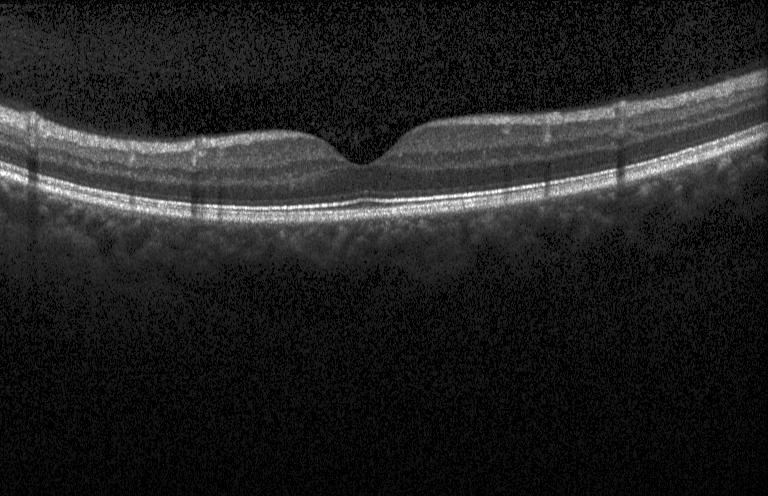
OCT finding: no choroidal neovascularization, no diabetic macular edema, and no drusen.